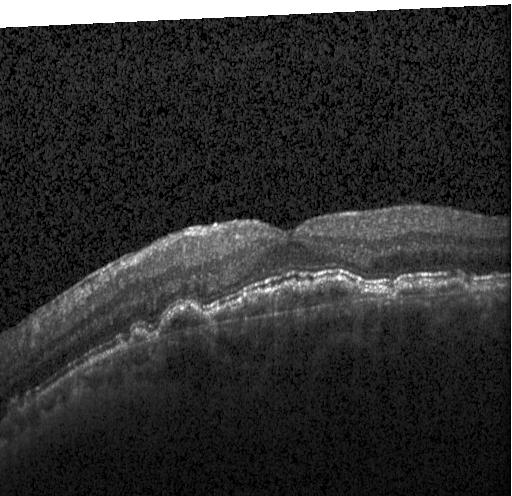

Spectral-domain OCT B-scan: CNV.